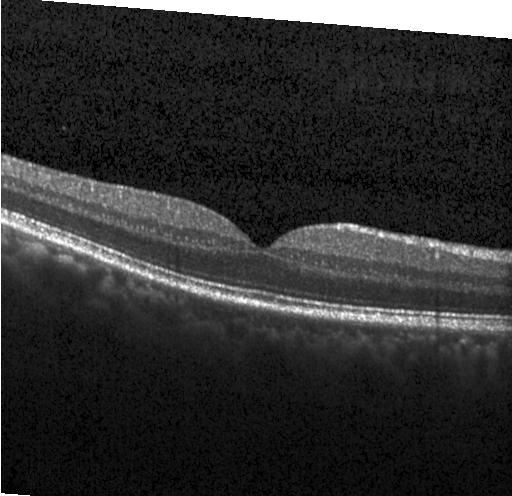 Impression: no evidence of choroidal neovascularization, diabetic macular edema, or drusen.